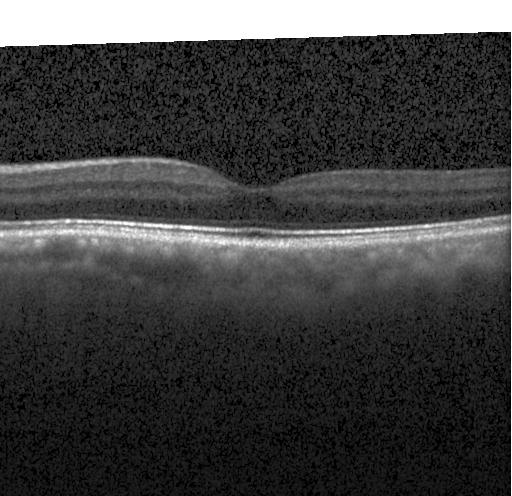
Macular scan, retinal OCT B-scan, Heidelberg Spectralis — This B-scan demonstrates no evidence of choroidal neovascularization, diabetic macular edema, or drusen.